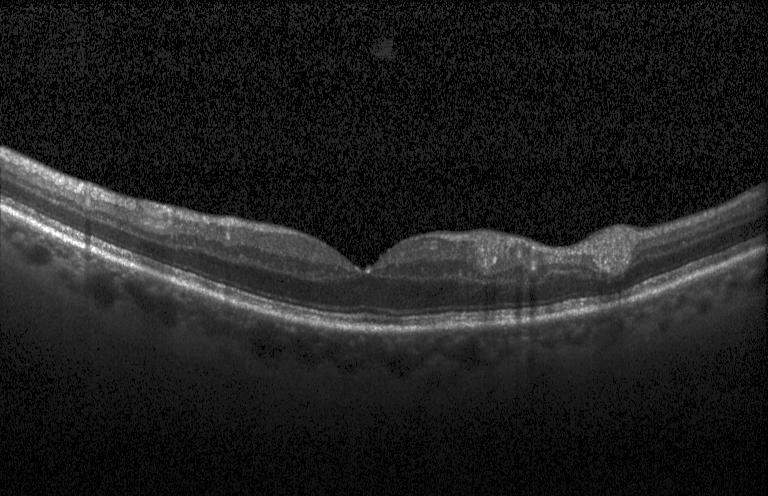
OCT line scan. Diagnosis: neither choroidal neovascularization, diabetic macular edema, nor drusen.